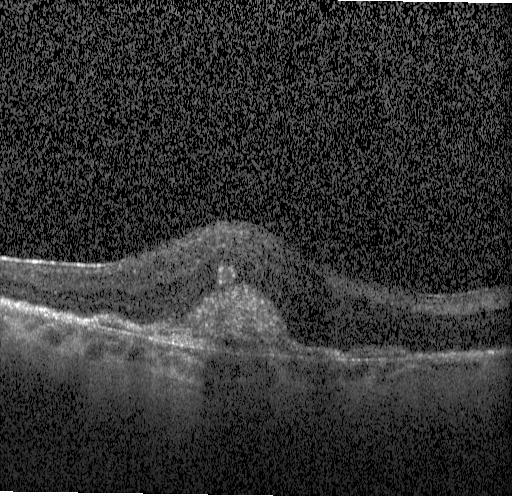
OCT finding: CNV.